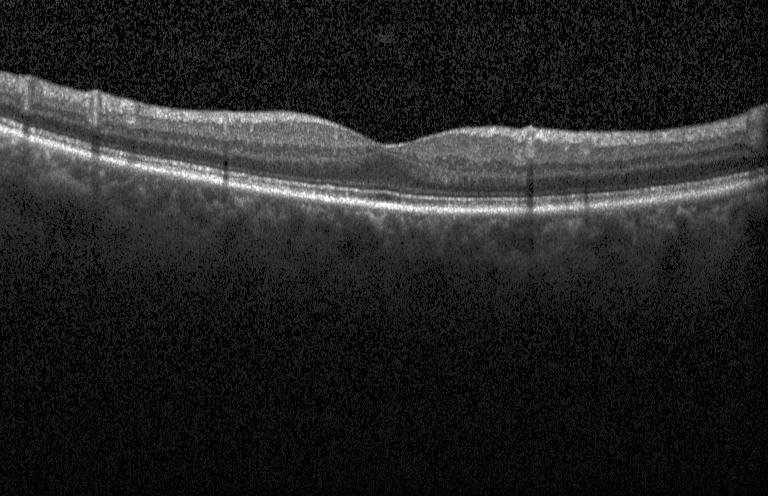 The scan shows no CNV, DME, or drusen.